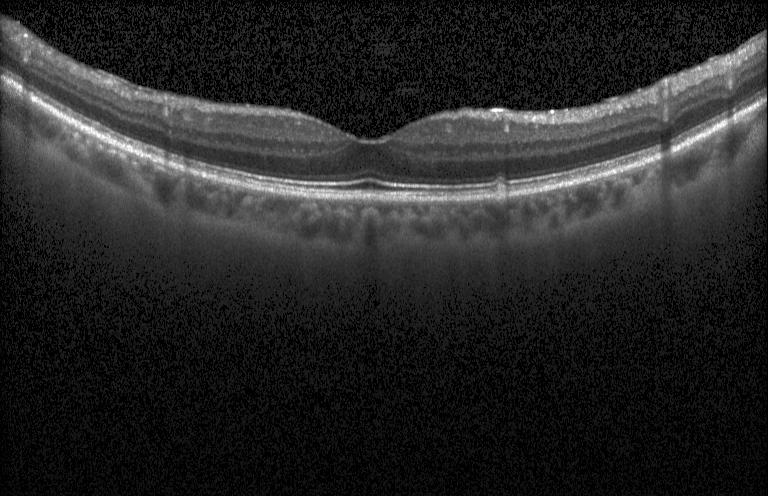

Instrument: Heidelberg Spectralis. Retinal OCT cross-section
Assessment: no evidence of choroidal neovascularization, diabetic macular edema, or drusen.